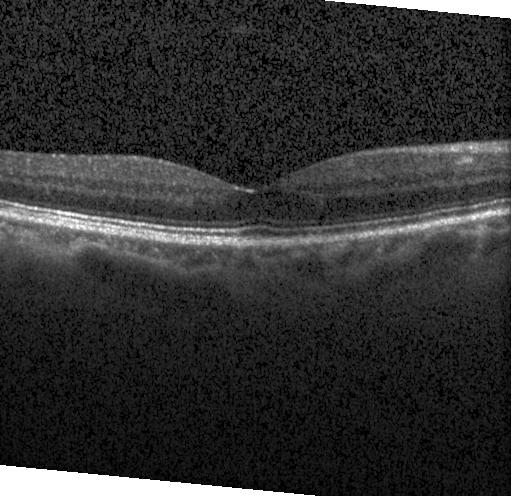 SD-OCT; OCT line scan
Impression: no CNV, DME, or drusen.